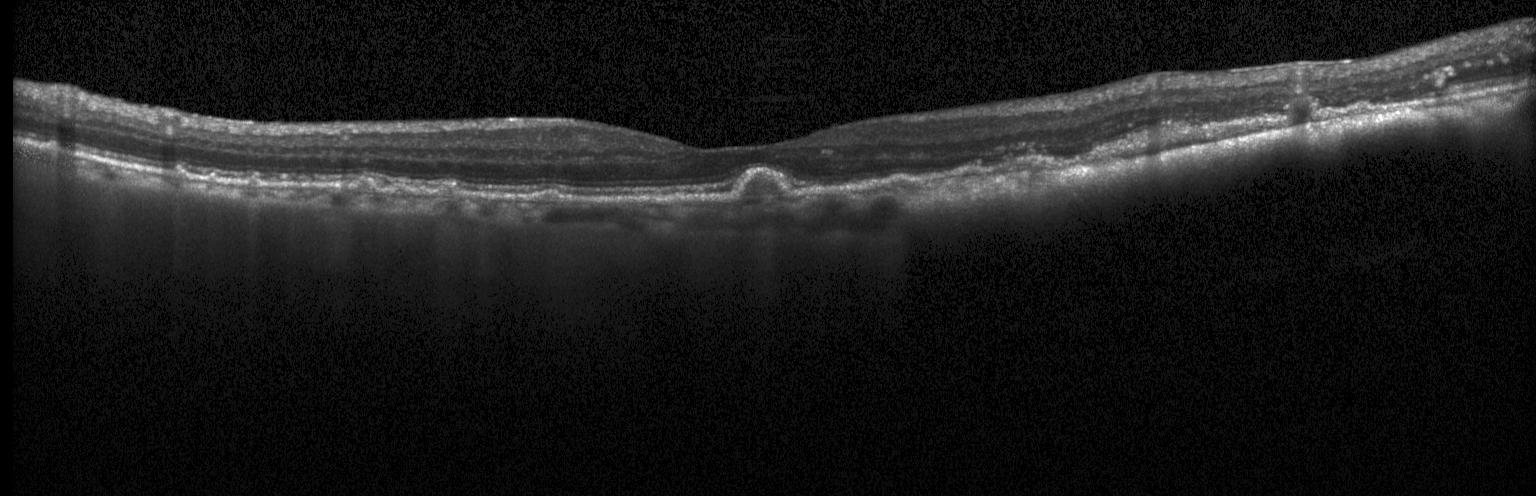 Finding: a choroidal neovascular membrane.